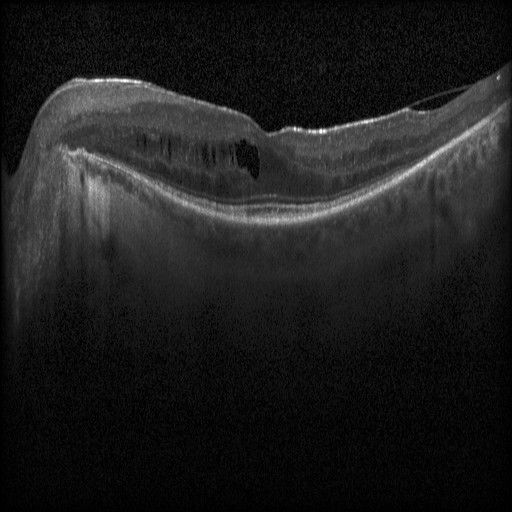

Impression: diabetic macular edema.